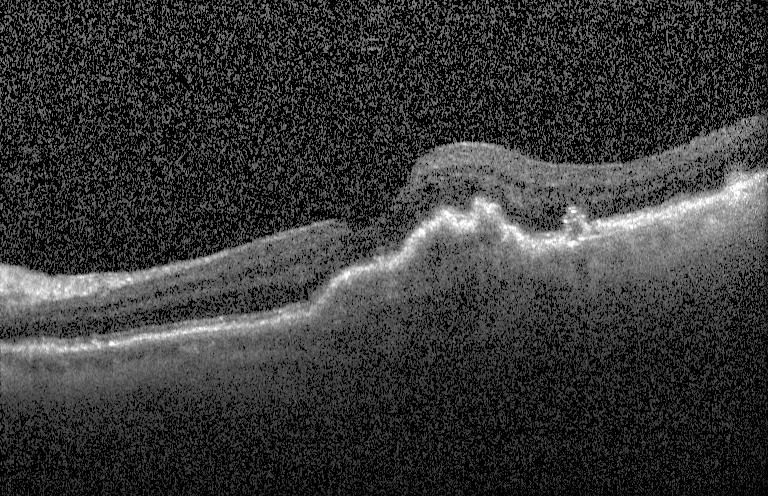

Optical coherence tomography scan · horizontal scan through the fovea · Heidelberg Spectralis
The scan shows choroidal neovascularization (CNV).